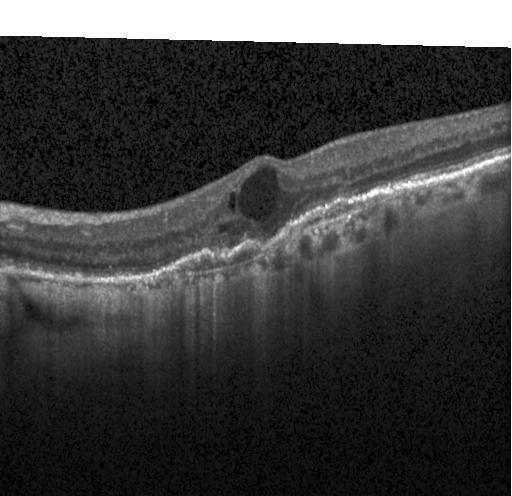
Retinal OCT B-scan — Finding: a choroidal neovascular membrane.